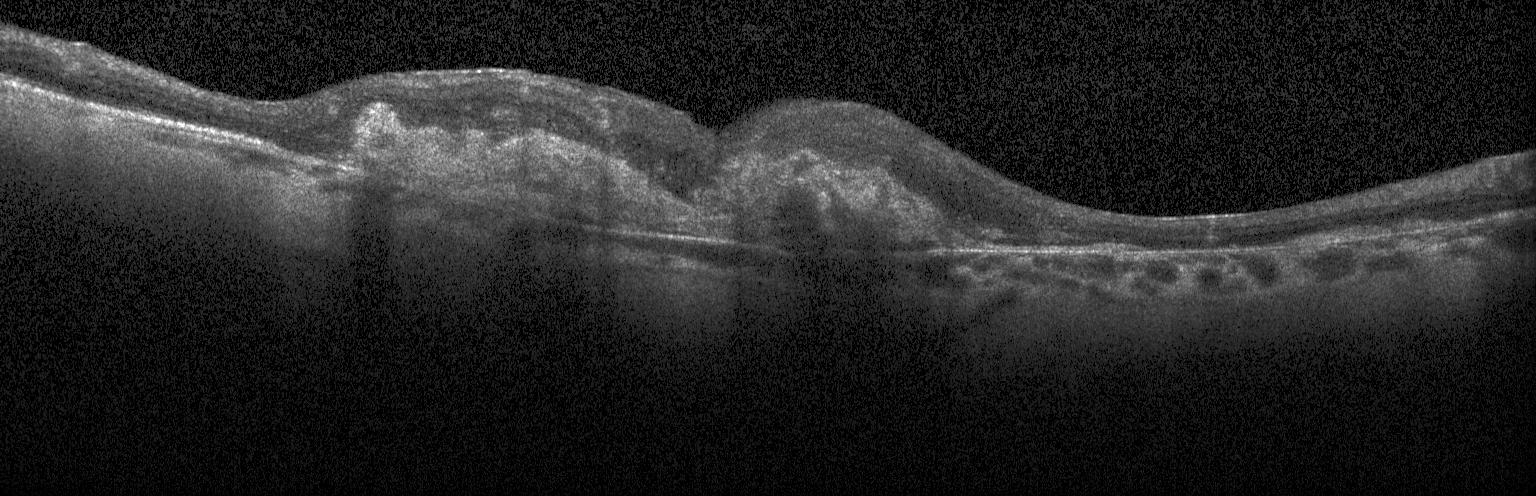
Impression: a choroidal neovascular membrane.